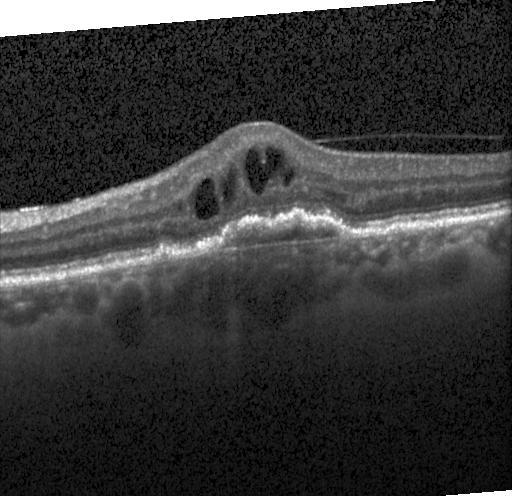
A choroidal neovascular membrane.